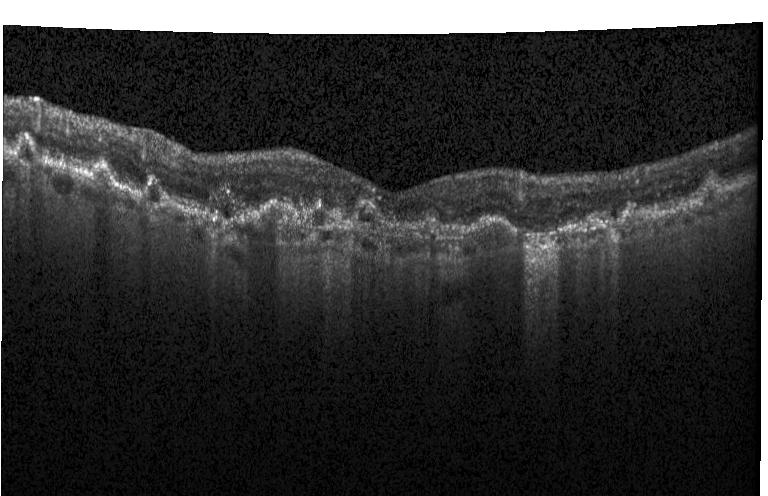 OCT scan showing choroidal neovascularization.